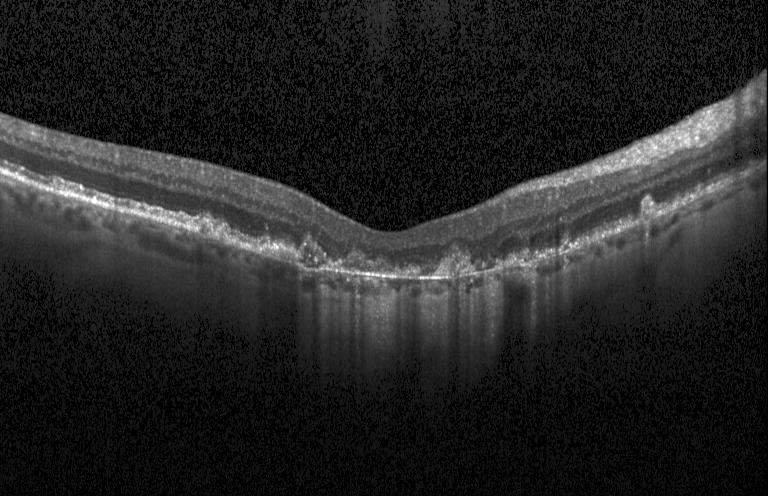
Through the macula; OCT line scan; SD-OCT. Finding: CNV.